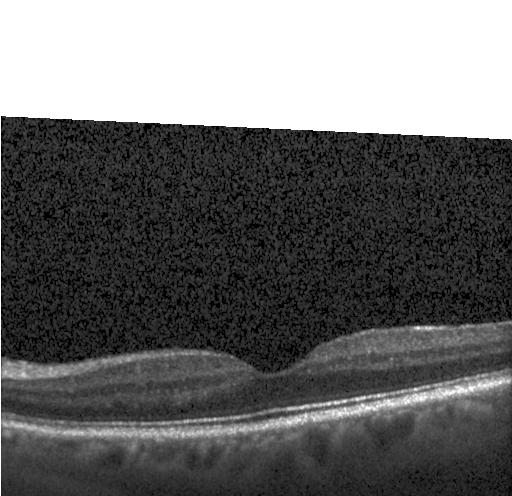
Optical coherence tomography B-scan
The scan shows no evidence of choroidal neovascularization, diabetic macular edema, or drusen.